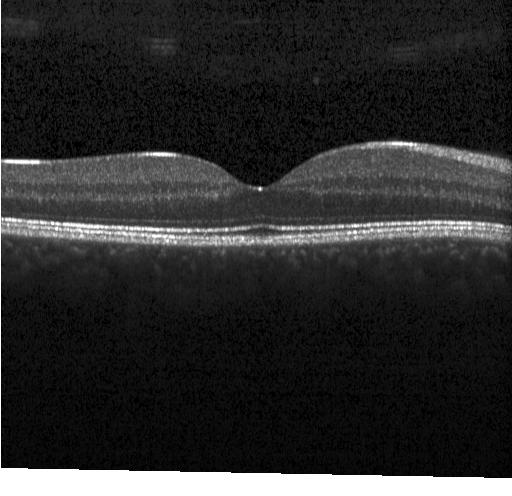

Impression: neither choroidal neovascularization, diabetic macular edema, nor drusen.